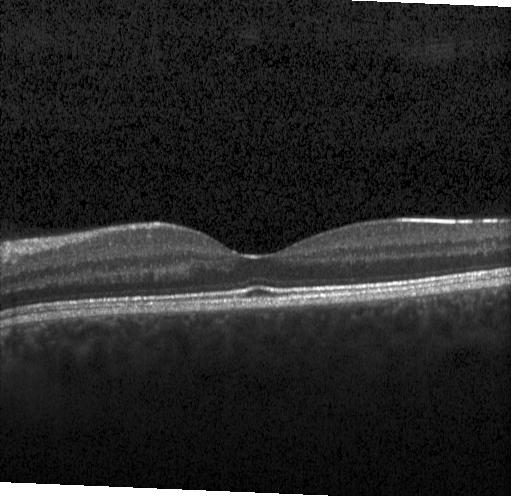
Optical coherence tomography scan · Heidelberg Spectralis OCT system · fovea-centered · spectral-domain OCT. Finding: no CNV, DME, or drusen.